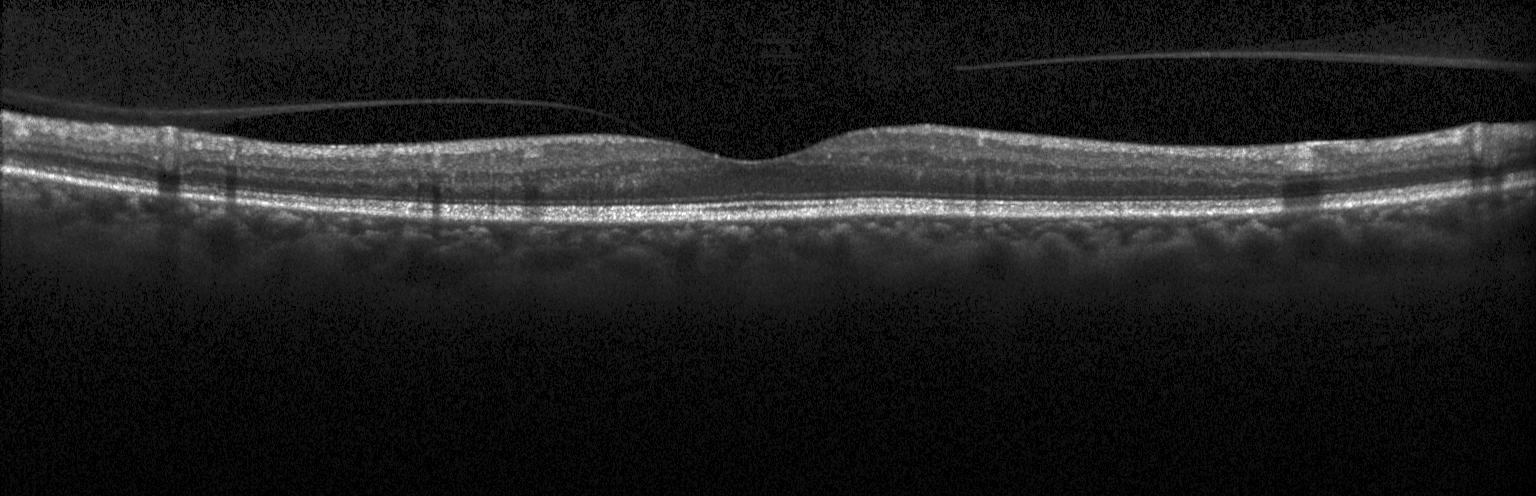
Optical coherence tomography B-scan. Dx: neither CNV, DME, nor drusen.